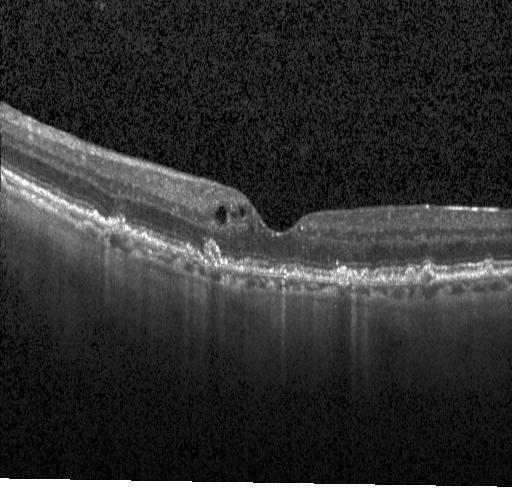
Spectral-domain optical coherence tomography. Through the macula. Retinal OCT B-scan. Heidelberg Spectralis.
Diagnosis: a choroidal neovascular membrane.